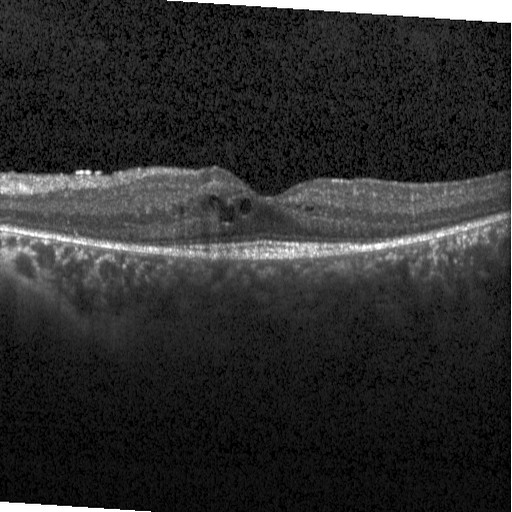
Impression: DME.